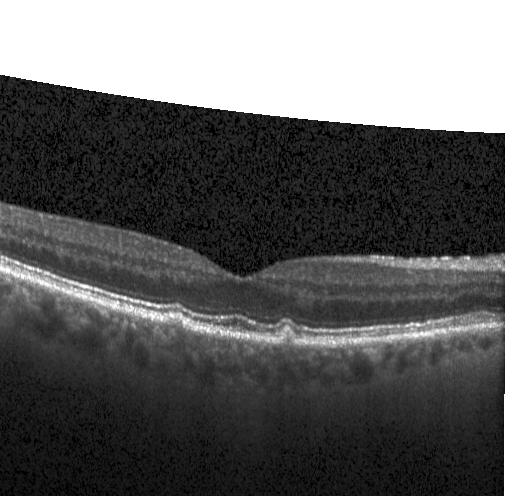

Optical coherence tomography B-scan. Diagnosis: multiple drusen.